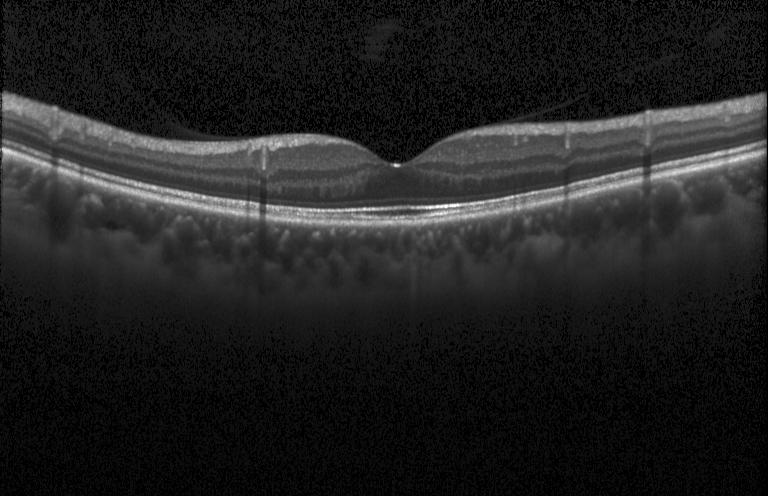

OCT line scan; through the macula; SD-OCT; instrument: Heidelberg Spectralis. Impression: no choroidal neovascularization, diabetic macular edema, or drusen.